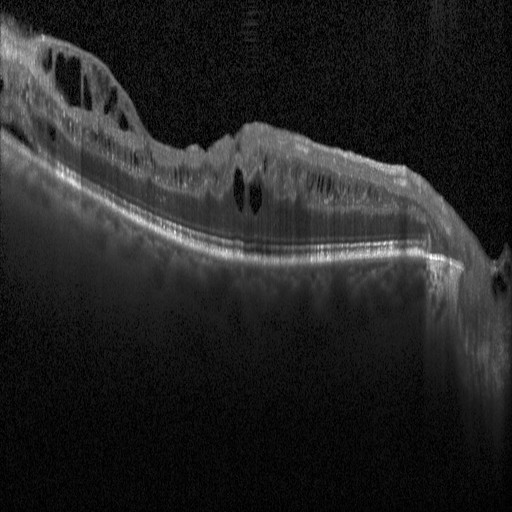 Retinal OCT cross-section showing diabetic macular edema.